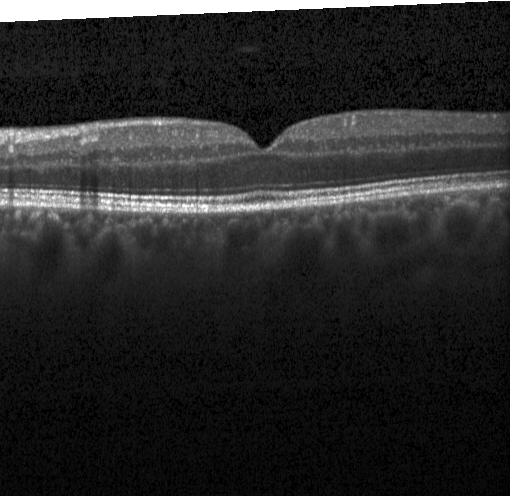 Optical coherence tomography scan. The scan shows no evidence of CNV, DME, or drusen.